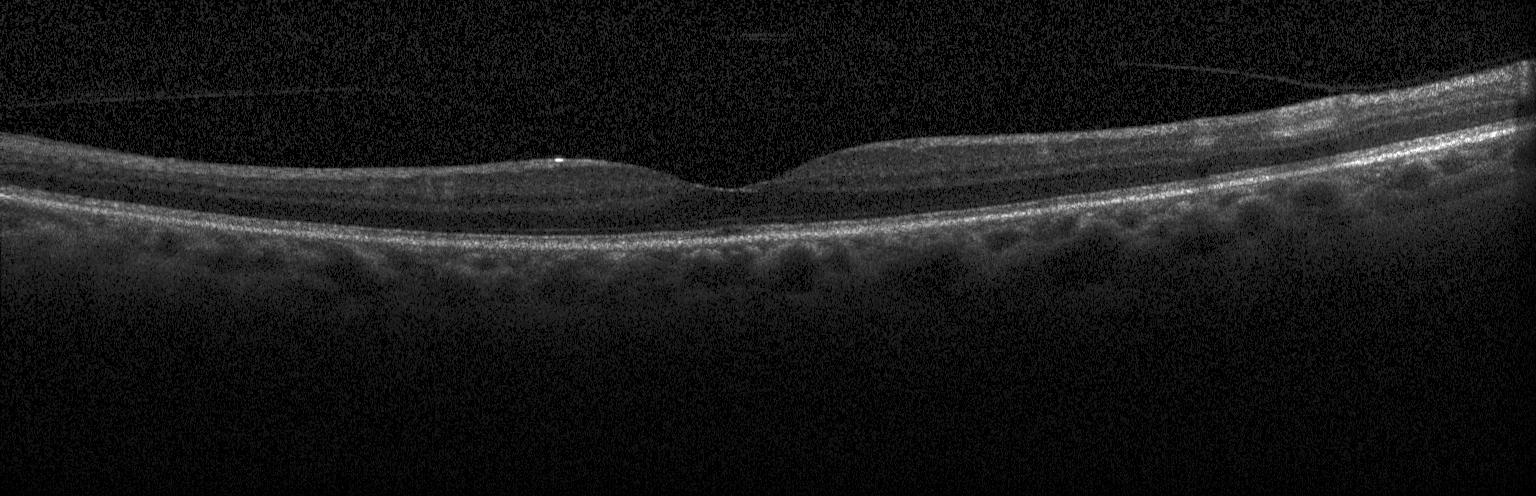 SD-OCT, fovea-centered, optical coherence tomography B-scan, acquired on a Heidelberg Spectralis.
Diagnosis: no choroidal neovascularization, no diabetic macular edema, and no drusen.